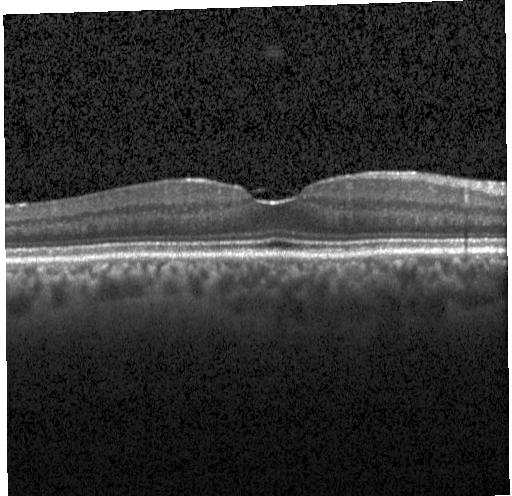 Retinal OCT B-scan; fovea-centered
Impression: no choroidal neovascularization, no diabetic macular edema, and no drusen.